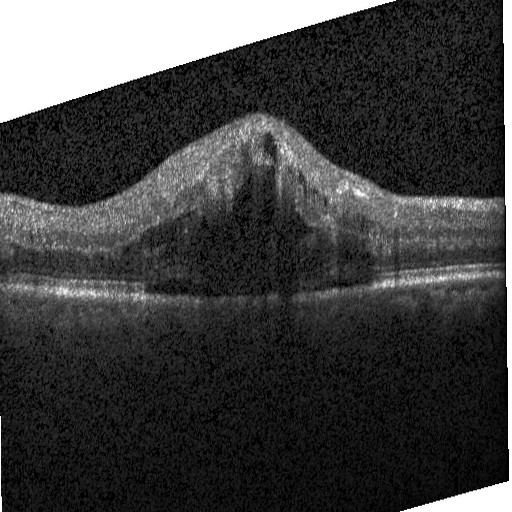

Spectral-domain optical coherence tomography. Acquired on a Heidelberg Spectralis. Retinal OCT B-scan — Assessment: DME.